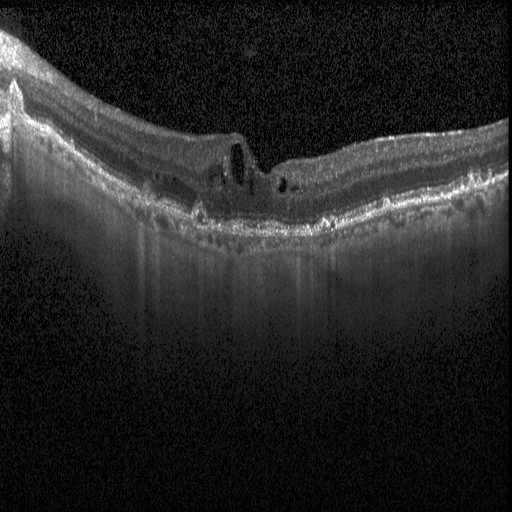

Retinal OCT B-scan. Impression: DME.